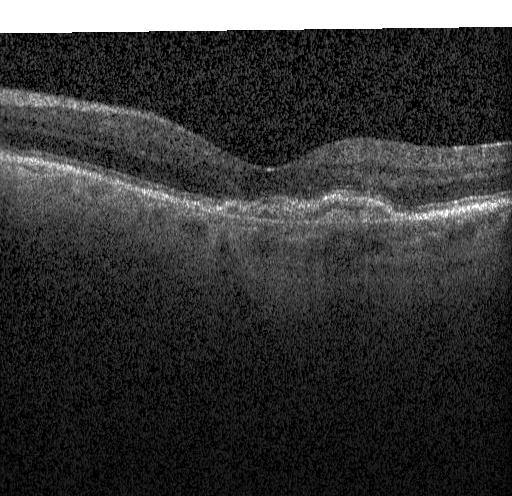 Diagnosis: choroidal neovascularization (CNV).